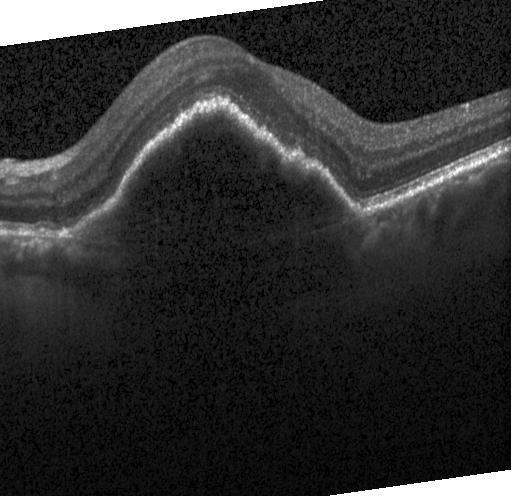

Impression: CNV.